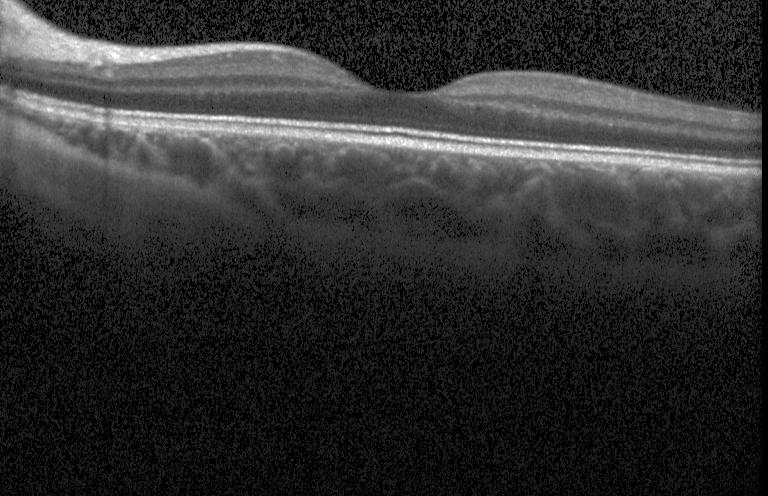 SD-OCT · through the macula · retinal OCT B-scan
The scan shows no choroidal neovascularization, diabetic macular edema, or drusen.